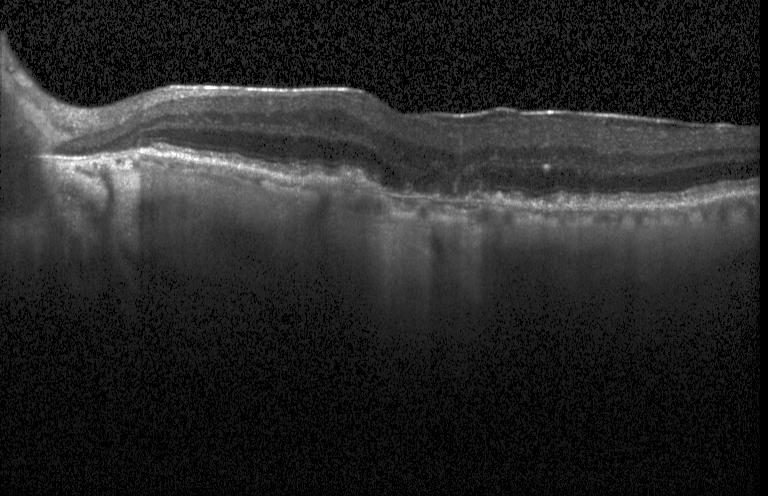

Heidelberg Spectralis; macular scan; spectral-domain optical coherence tomography; OCT line scan.
Finding: CNV.